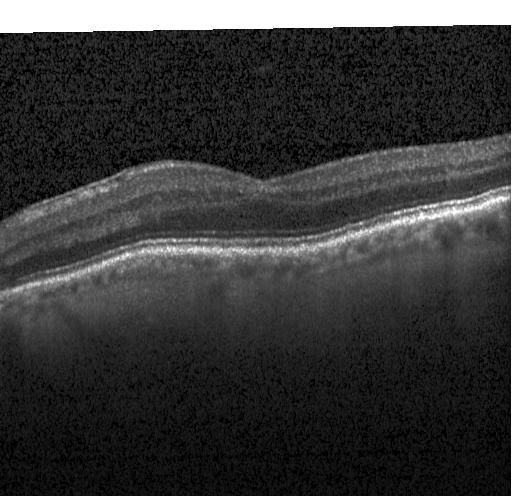 Spectral-domain OCT B-scan: neither CNV, DME, nor drusen.